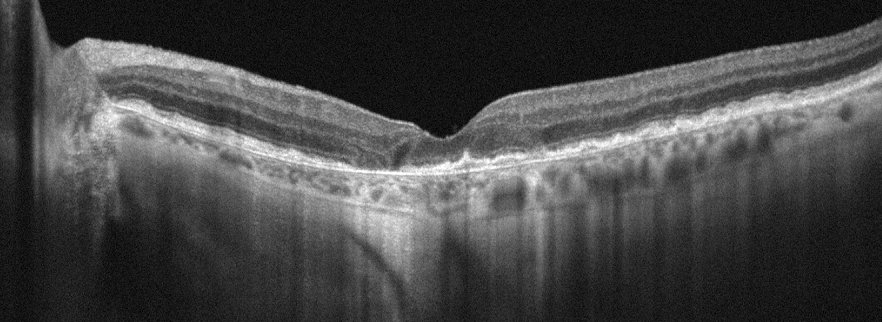 Retinal OCT cross-section · oculus sinister
Impression: AMD.